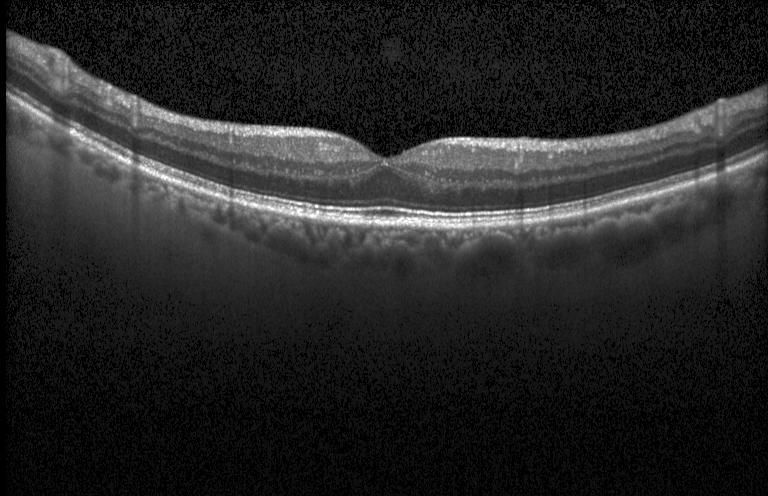 Impression: no choroidal neovascularization, diabetic macular edema, or drusen.